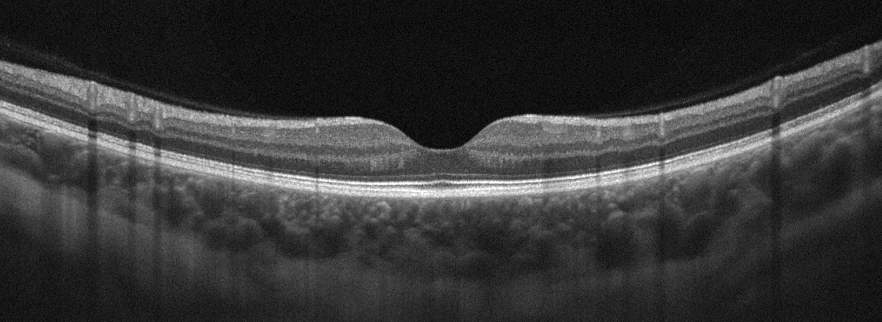 Right eye; OCT line scan; Optovue Avanti RTVue XR; fovea-centered
No evidence of AMD, DME, ERM, RAO, RVO, or VID.